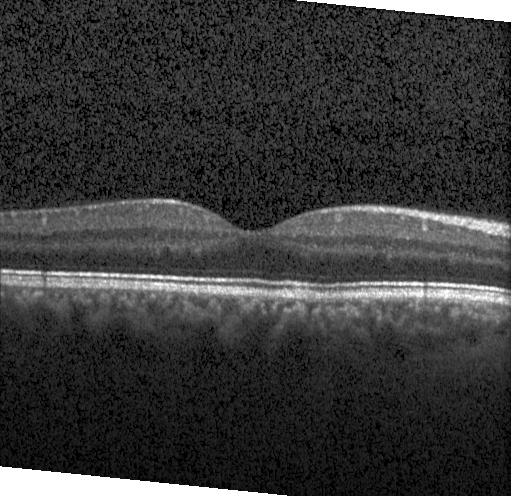 Diagnosis: no evidence of choroidal neovascularization, diabetic macular edema, or drusen.